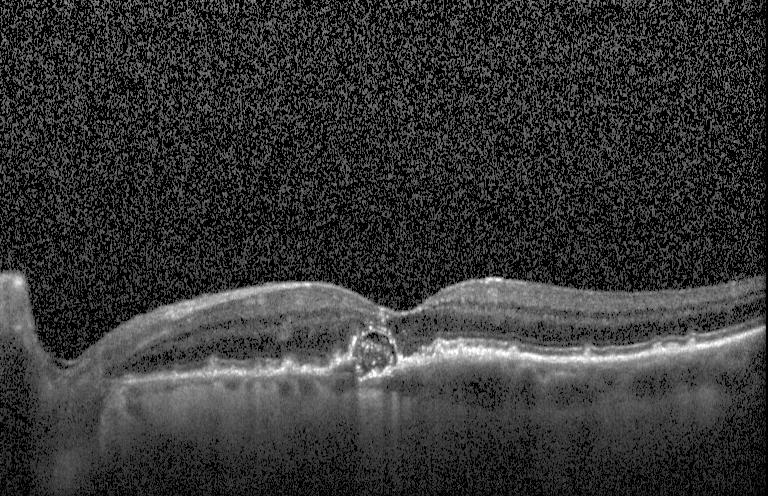
OCT line scan. SD-OCT. Assessment: a choroidal neovascular membrane.